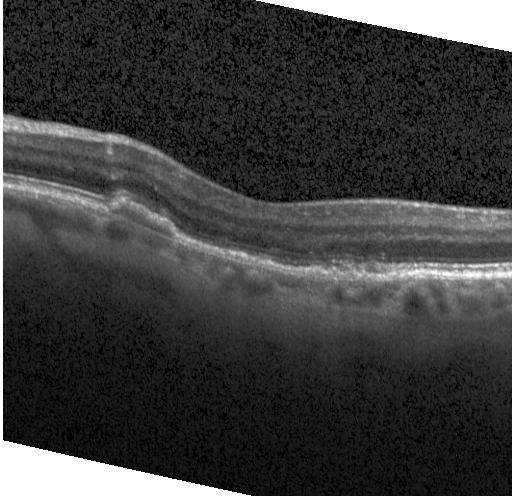
SD-OCT · OCT line scan · through the macula · instrument: Heidelberg Spectralis
Macular OCT: choroidal neovascularization.